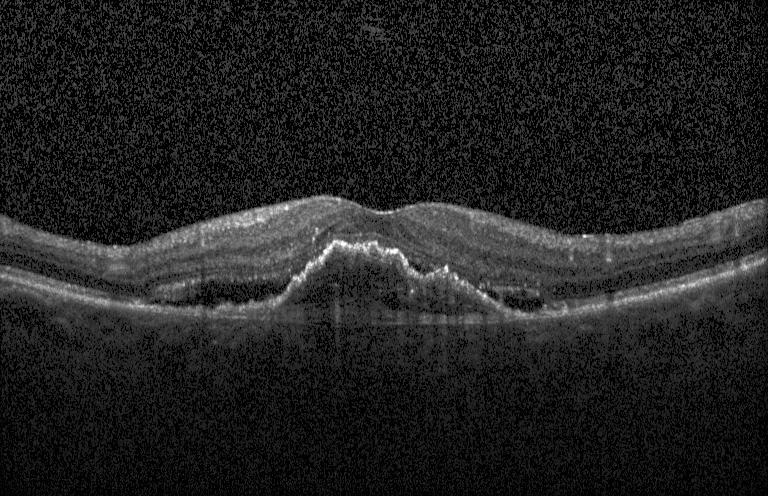

Retinal OCT cross-section, instrument: Heidelberg Spectralis, horizontal scan through the fovea, spectral-domain optical coherence tomography
Choroidal neovascularization (CNV).